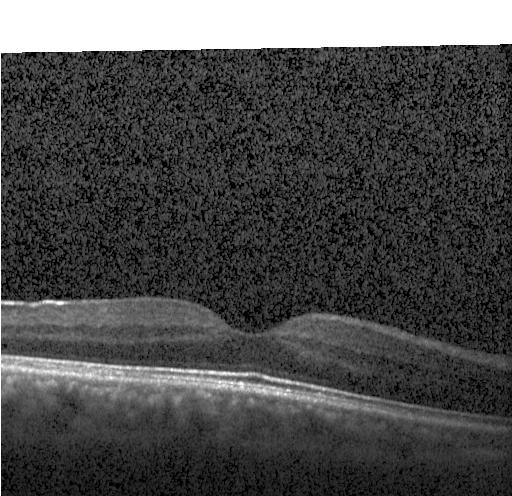
Macular OCT demonstrating neither choroidal neovascularization, diabetic macular edema, nor drusen.